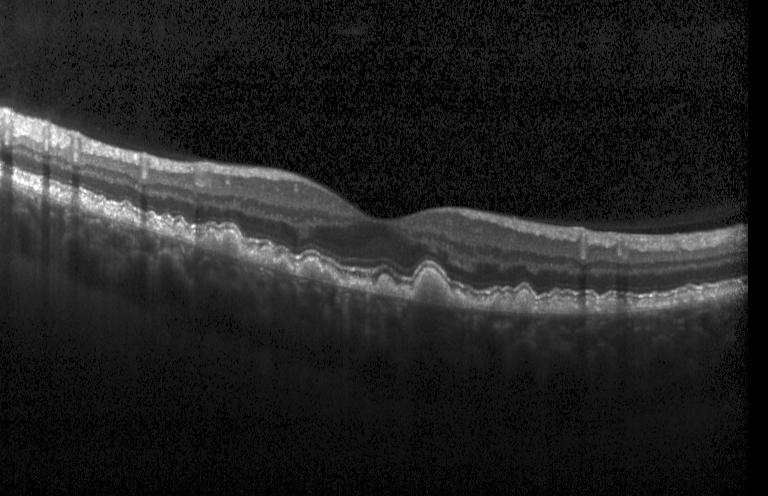
Acquired on a Heidelberg Spectralis · horizontal scan through the fovea · spectral-domain OCT · retinal OCT cross-section
Dx: sub-RPE drusenoid deposits.